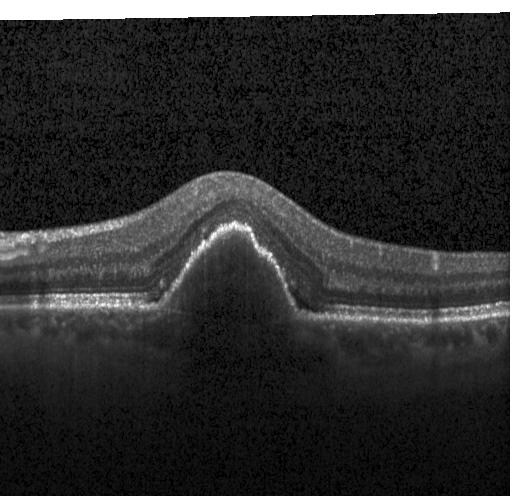

OCT line scan. Spectral-domain optical coherence tomography — Dx: CNV.